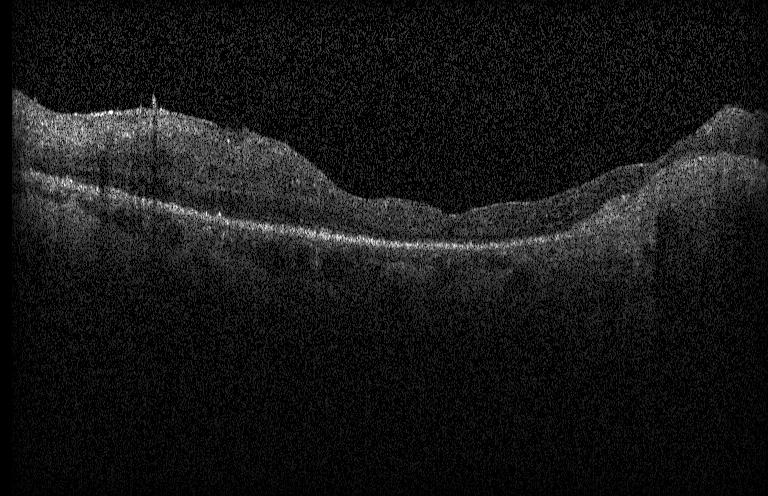

Centered on the fovea; retinal OCT cross-section; Heidelberg Spectralis. Finding: CNV.